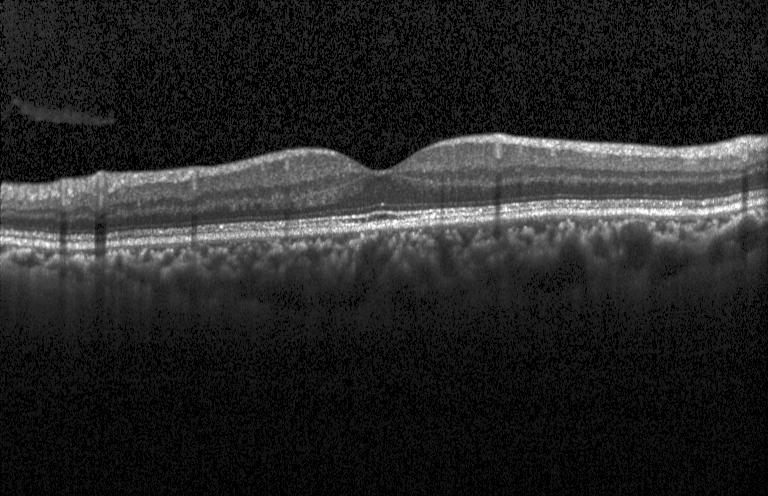
The scan shows no evidence of CNV, DME, or drusen.